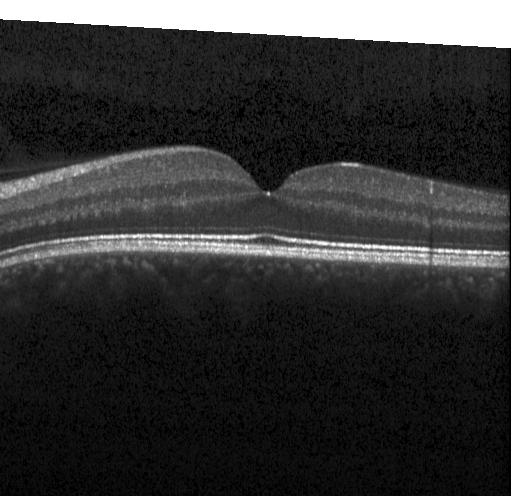

Retinal OCT B-scan, fovea-centered
Diagnosis: no evidence of choroidal neovascularization, diabetic macular edema, or drusen.